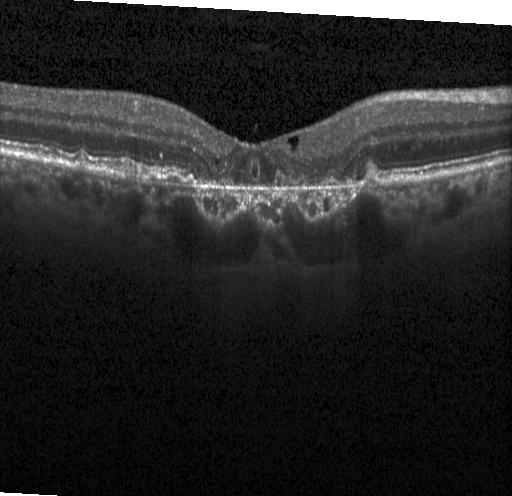
Macular OCT: a choroidal neovascular membrane.